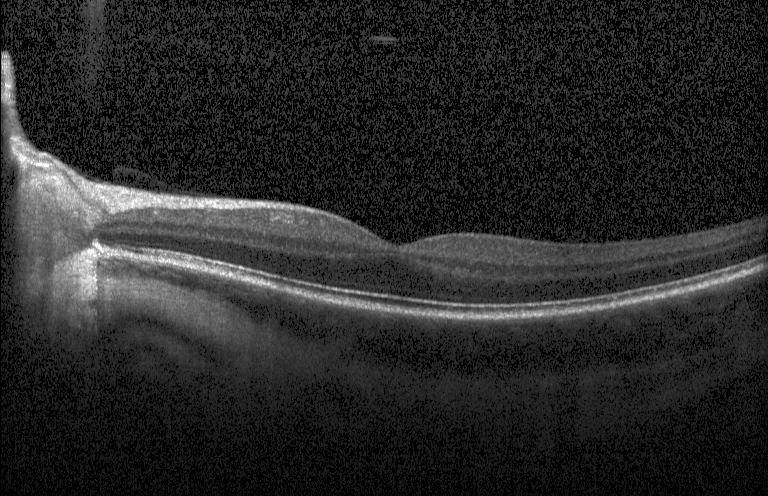

Optical coherence tomography B-scan
This B-scan demonstrates no choroidal neovascularization, no diabetic macular edema, and no drusen.